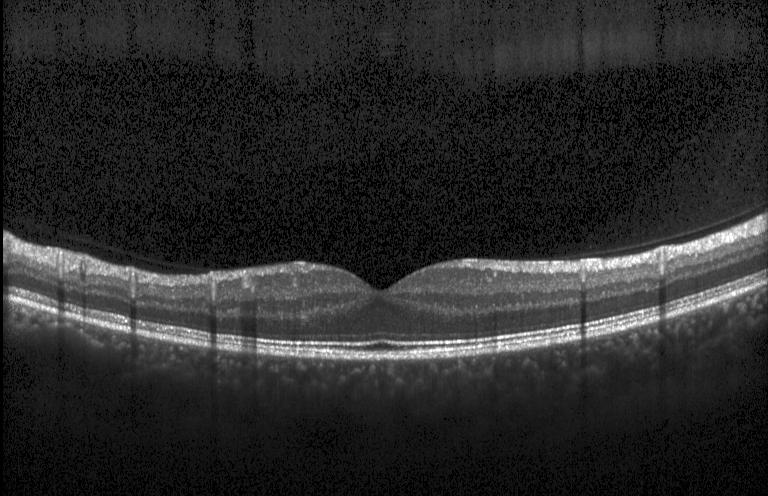 Macular scan · retinal OCT cross-section · SD-OCT · instrument: Heidelberg Spectralis — Impression: no CNV, DME, or drusen.